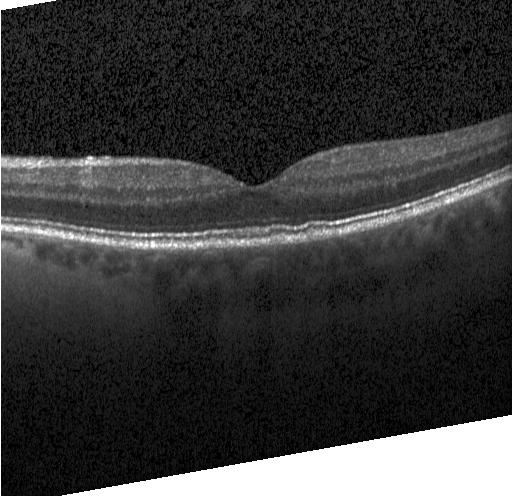 Fovea-centered. Heidelberg Spectralis. Optical coherence tomography scan. Spectral-domain OCT. Finding: multiple drusen.